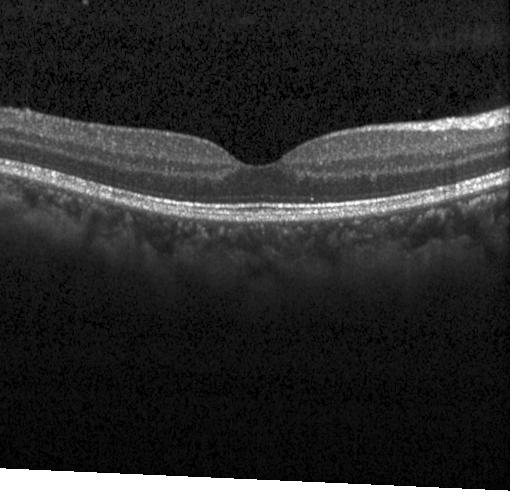 Optical coherence tomography B-scan — Finding: no evidence of choroidal neovascularization, diabetic macular edema, or drusen.